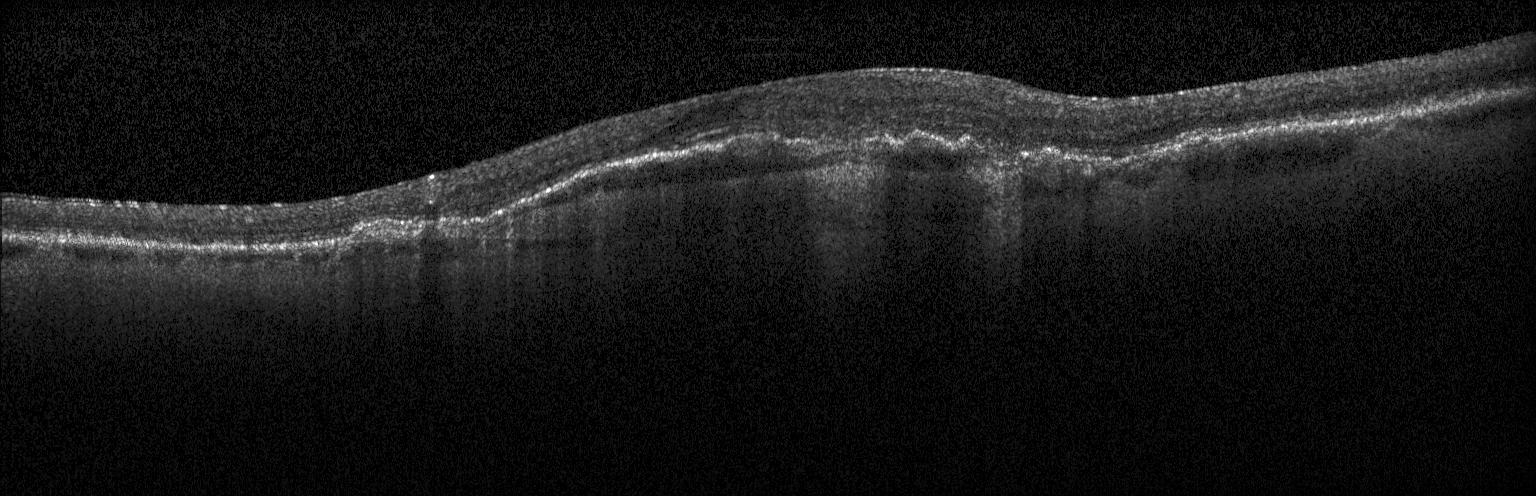
Diagnosis: a choroidal neovascular membrane.